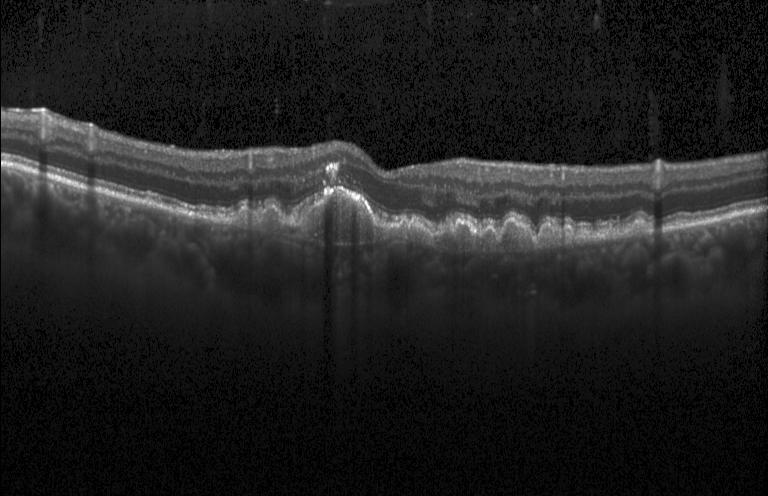
Retinal OCT cross-section showing a choroidal neovascular membrane.